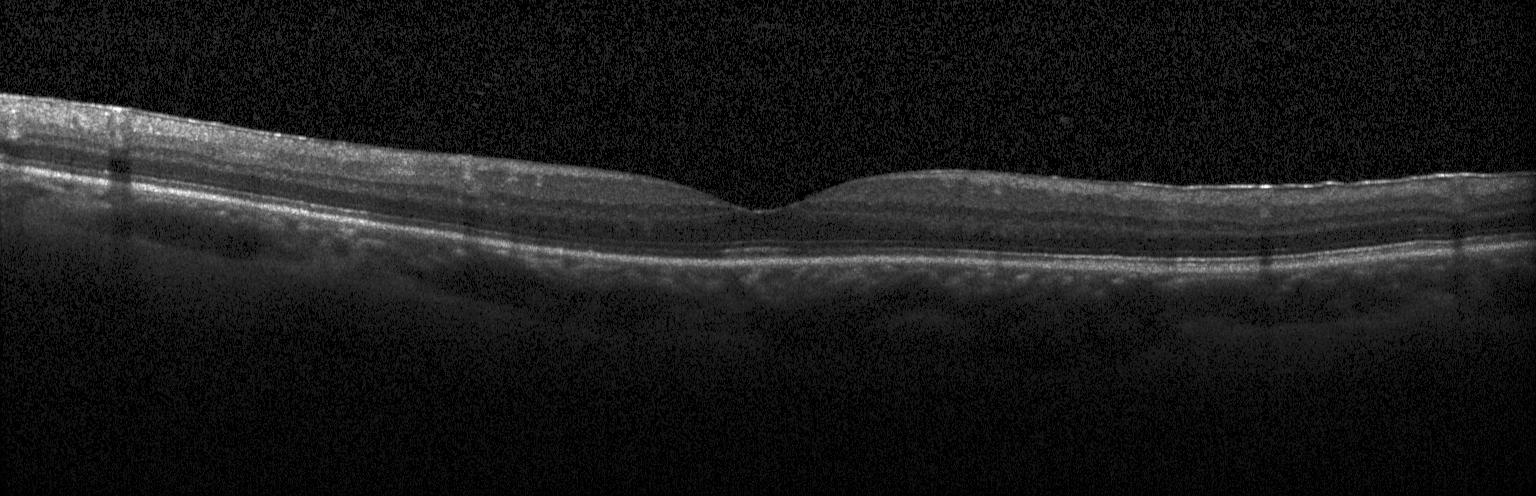 Finding: no choroidal neovascularization, no diabetic macular edema, and no drusen.